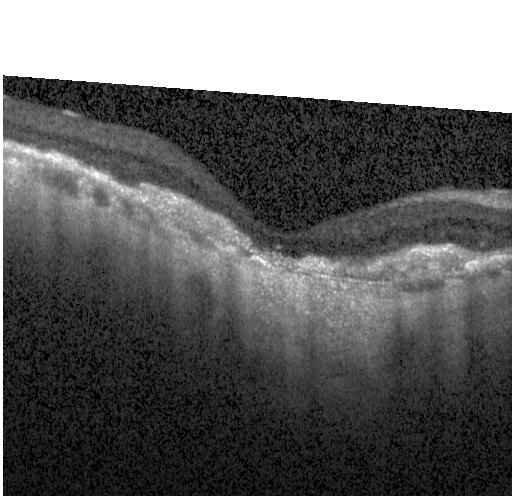 OCT line scan. Instrument: Heidelberg Spectralis
A choroidal neovascular membrane.